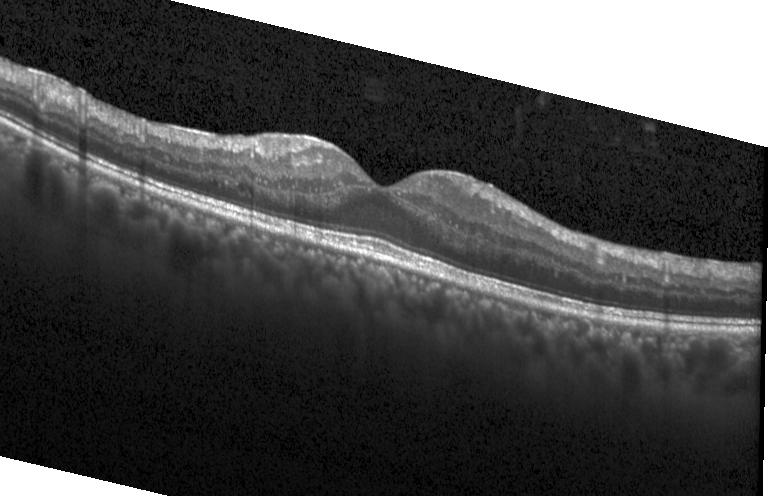 Spectral-domain optical coherence tomography. Retinal OCT B-scan. Instrument: Heidelberg Spectralis. Centered on the fovea.
Dx: no choroidal neovascularization, diabetic macular edema, or drusen.